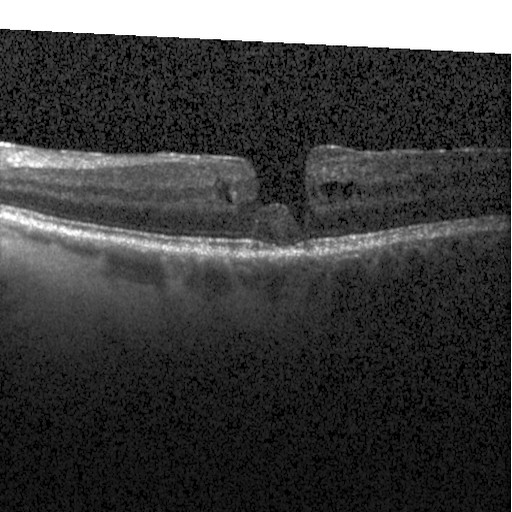

Retinal OCT B-scan.
Diagnosis: DME.